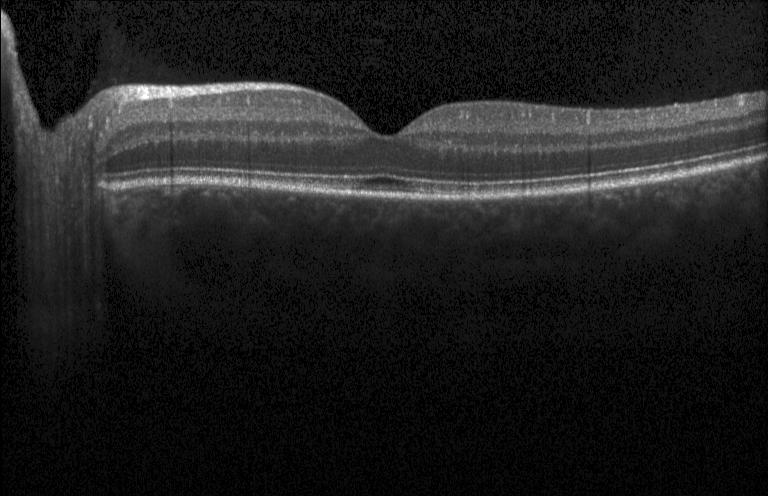
Acquired on a Heidelberg Spectralis · horizontal scan through the fovea · optical coherence tomography scan · spectral-domain optical coherence tomography
Impression: no choroidal neovascularization, diabetic macular edema, or drusen.